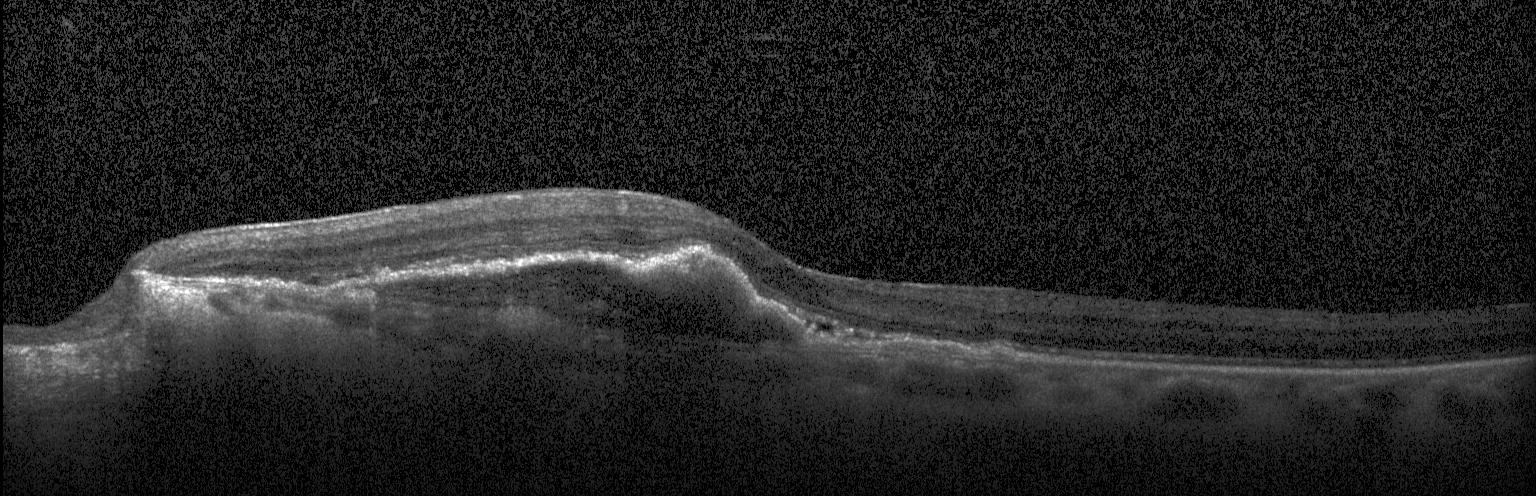 This B-scan demonstrates choroidal neovascularization.